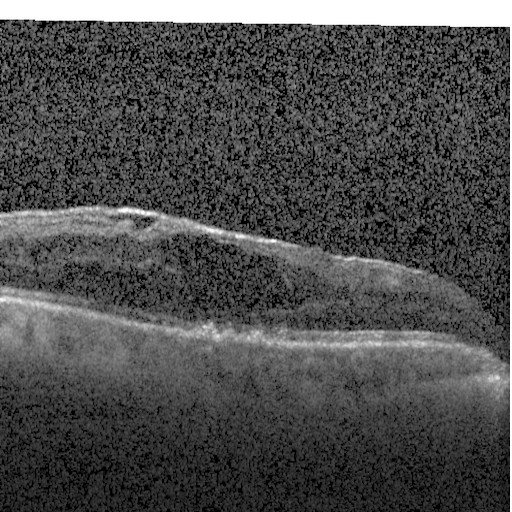

Fovea-centered · SD-OCT · optical coherence tomography scan · Heidelberg Spectralis
Dx: DME.